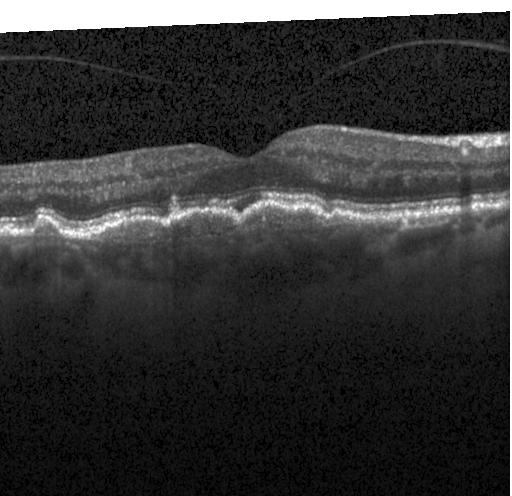

Optical coherence tomography B-scan. The scan shows choroidal neovascularization.